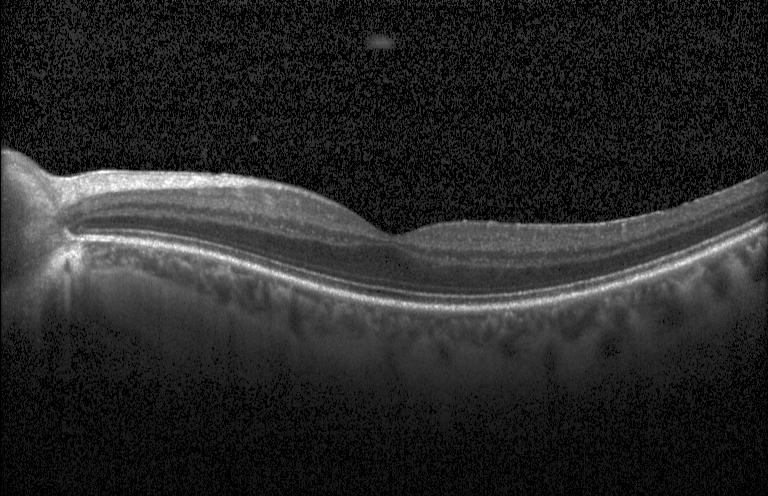

Through the macula · retinal OCT B-scan · spectral-domain optical coherence tomography.
Dx: no choroidal neovascularization, no diabetic macular edema, and no drusen.